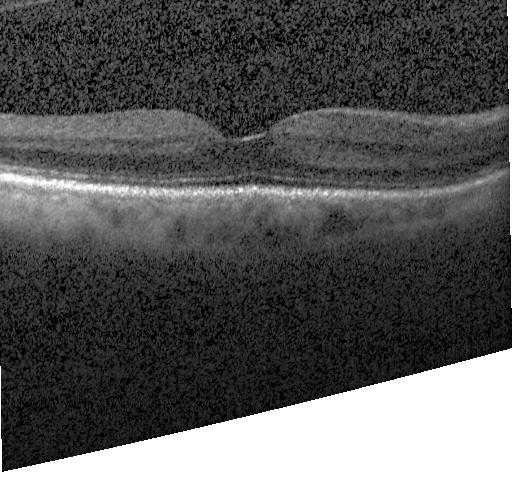

Spectral-domain optical coherence tomography; horizontal scan through the fovea; optical coherence tomography B-scan — Assessment: neither choroidal neovascularization, diabetic macular edema, nor drusen.